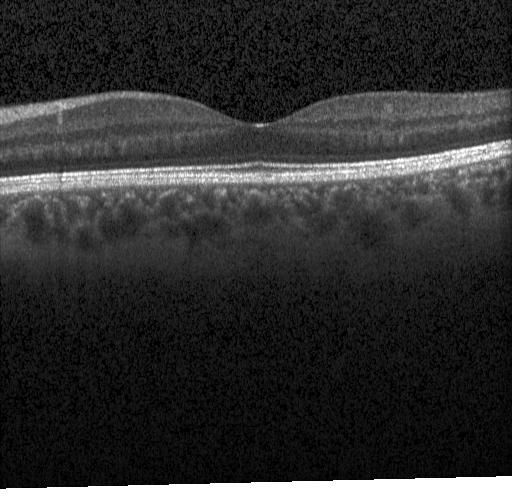
Assessment: no choroidal neovascularization, no diabetic macular edema, and no drusen.